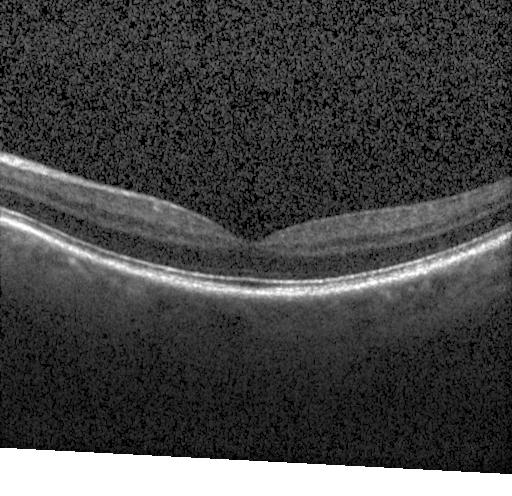

Heidelberg Spectralis OCT system. Retinal OCT B-scan.
Diagnosis: neither CNV, DME, nor drusen.